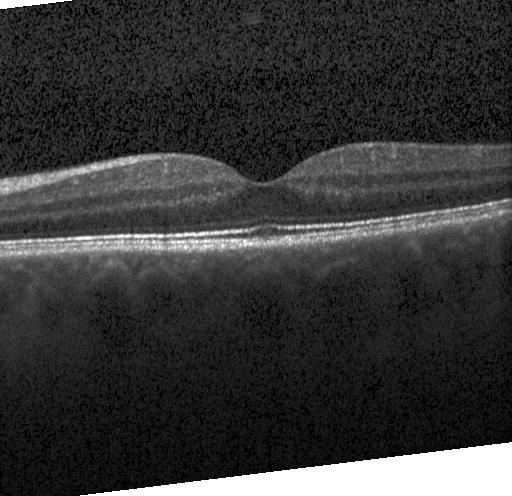
The scan shows no evidence of CNV, DME, or drusen.